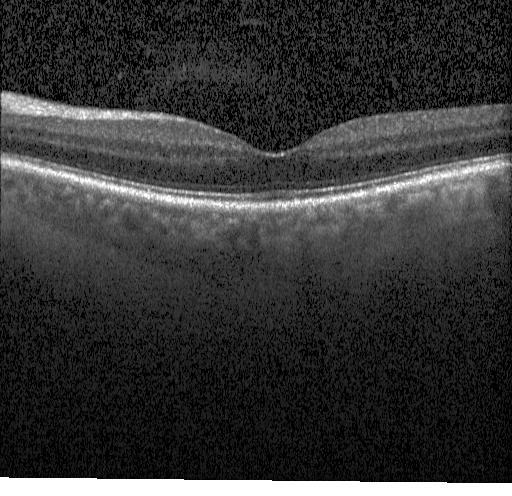
Spectral-domain OCT, optical coherence tomography B-scan, instrument: Heidelberg Spectralis, through the macula. Macular OCT: no choroidal neovascularization, diabetic macular edema, or drusen.